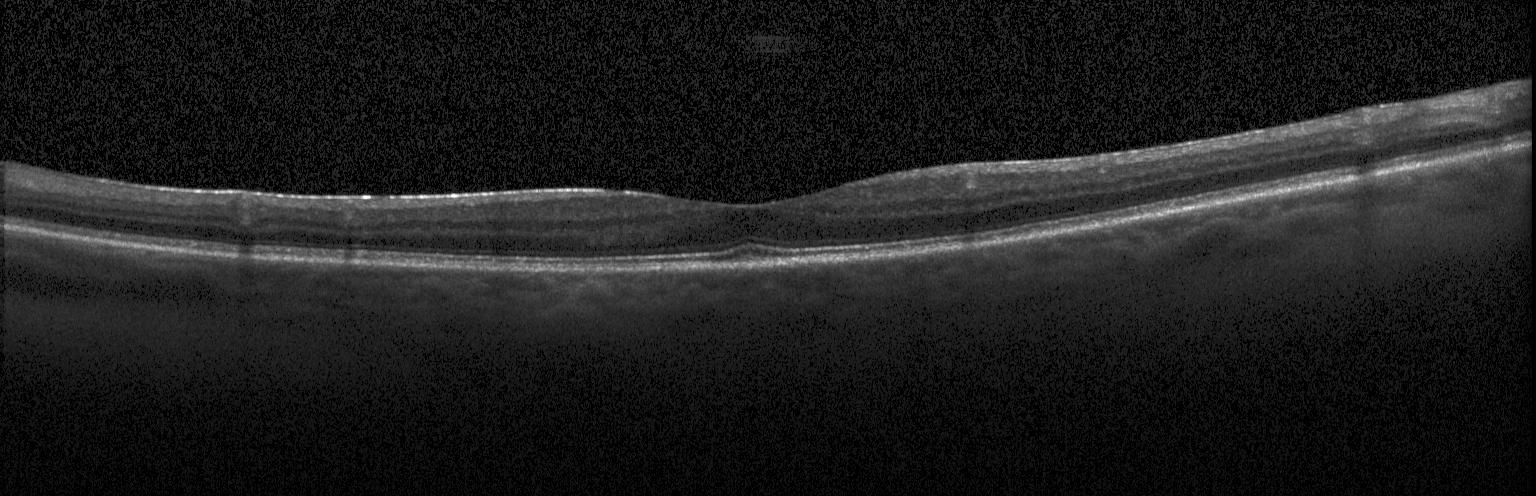 Optical coherence tomography B-scan; Heidelberg Spectralis OCT system
Dx: no evidence of CNV, DME, or drusen.